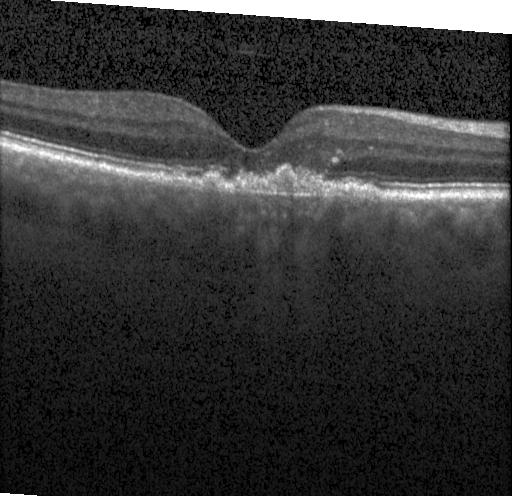 OCT line scan · through the macula · spectral-domain OCT. Finding: a choroidal neovascular membrane.